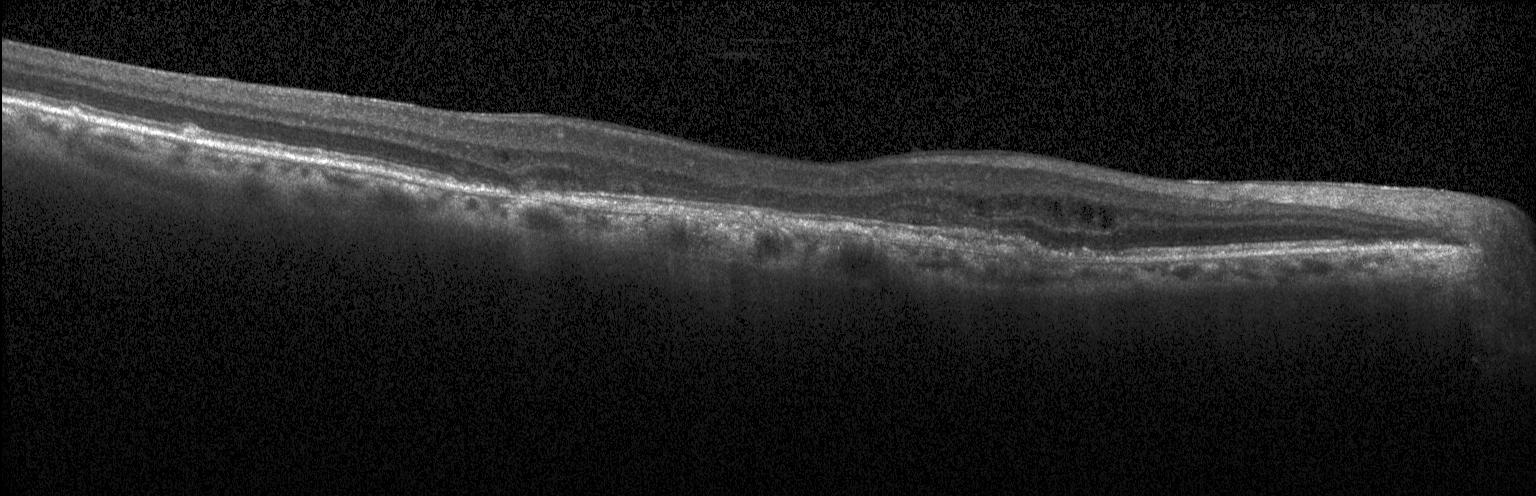 Macular OCT: a choroidal neovascular membrane.